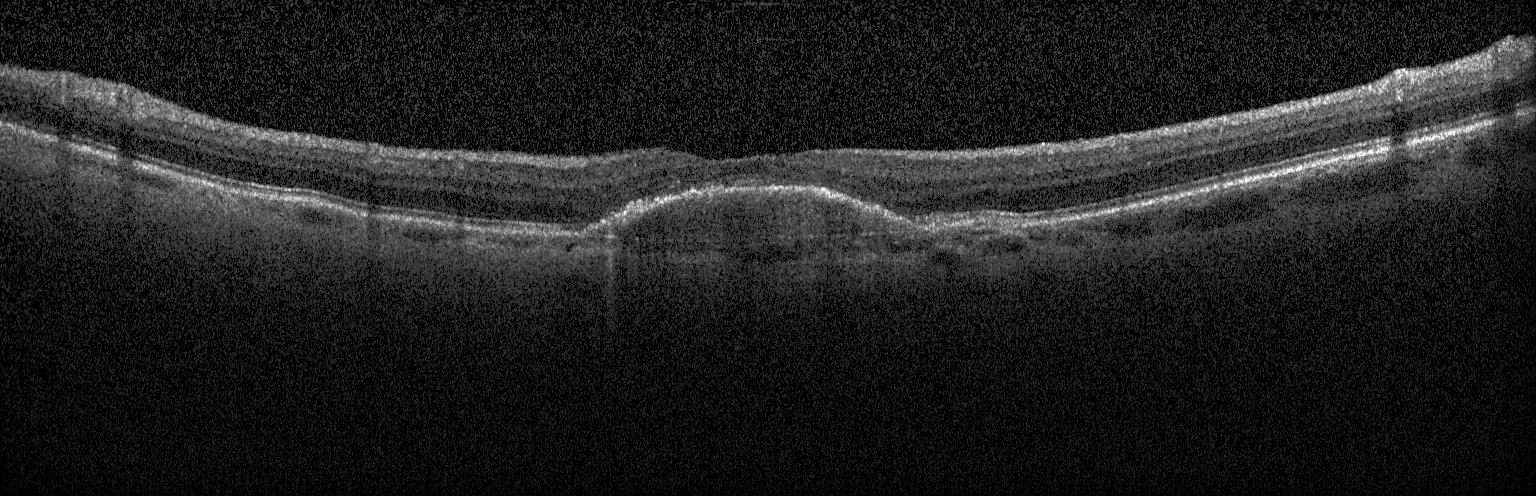

Centered on the fovea · optical coherence tomography scan · spectral-domain OCT · acquired on a Heidelberg Spectralis.
This B-scan demonstrates a choroidal neovascular membrane.